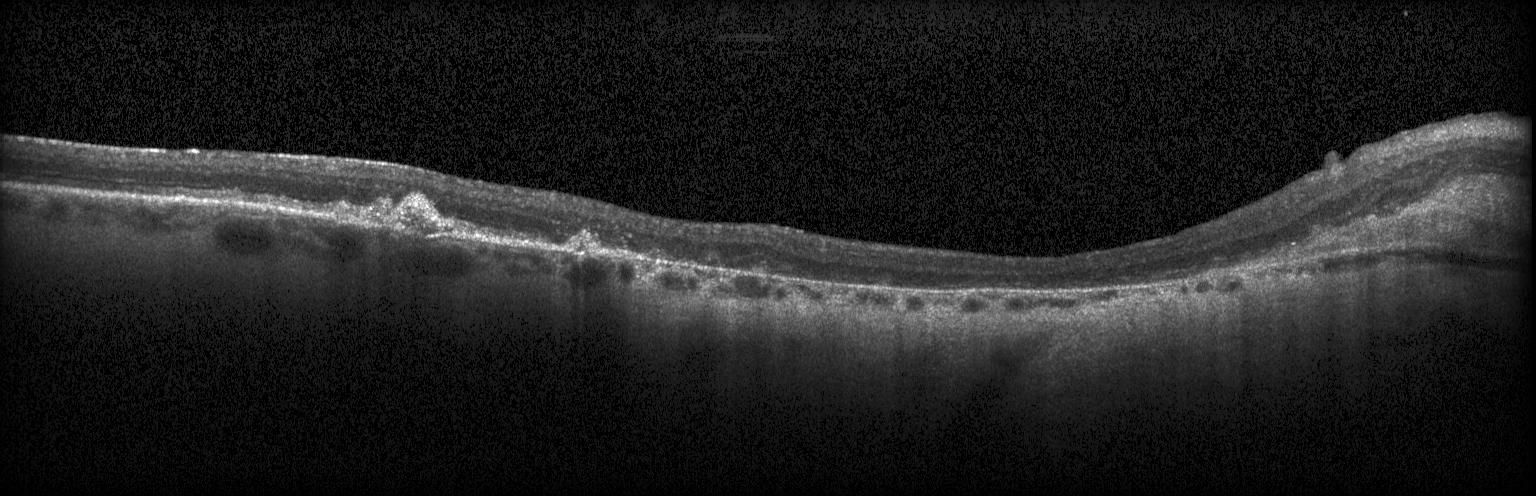

This B-scan demonstrates choroidal neovascularization.